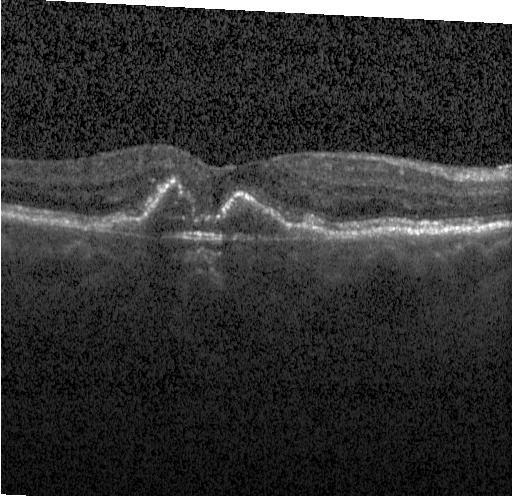 Optical coherence tomography B-scan. SD-OCT — Diagnosis: choroidal neovascularization (CNV).